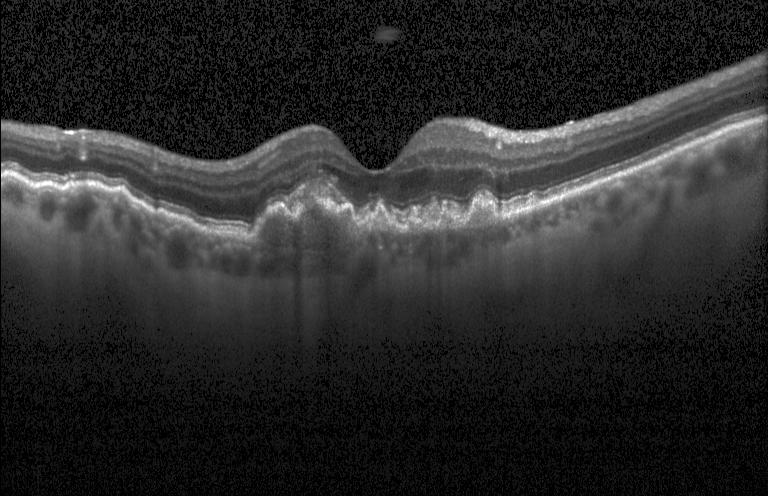

Optical coherence tomography scan.
The scan shows CNV.